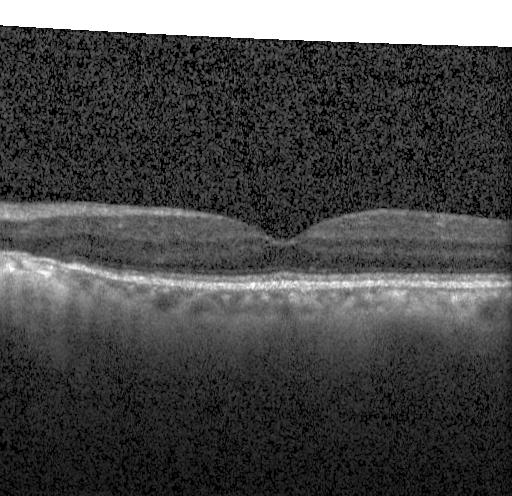 Retinal OCT cross-section.
No choroidal neovascularization, diabetic macular edema, or drusen.